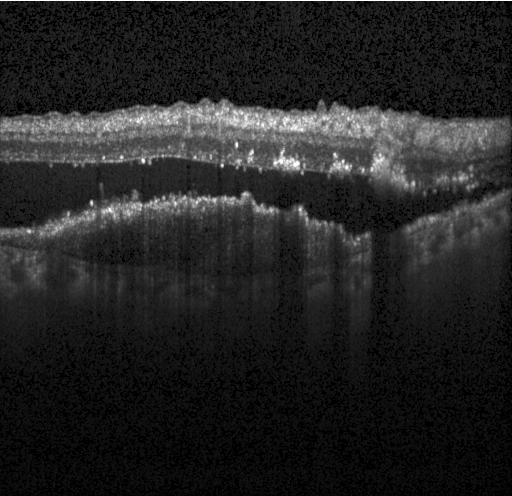

Assessment: a choroidal neovascular membrane.